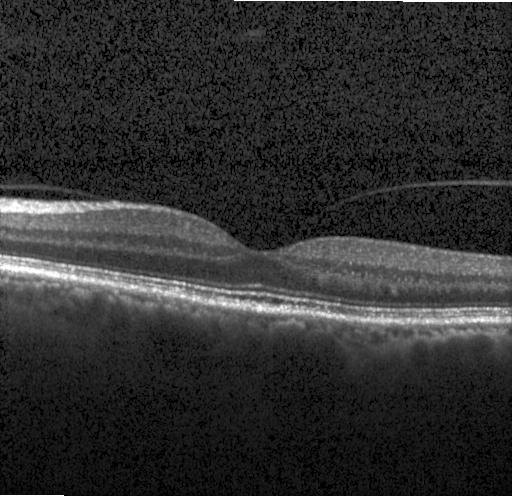

OCT finding: no evidence of choroidal neovascularization, diabetic macular edema, or drusen.